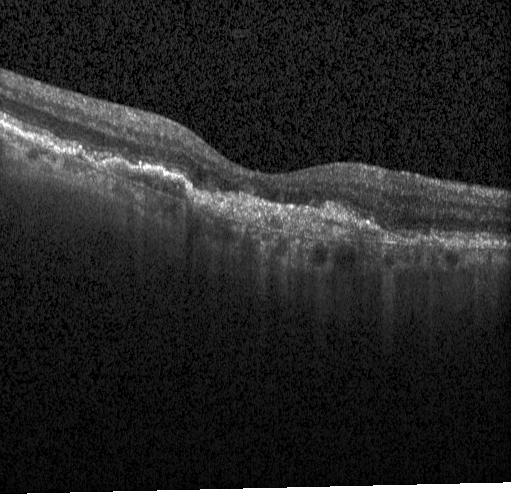
Impression: a choroidal neovascular membrane.